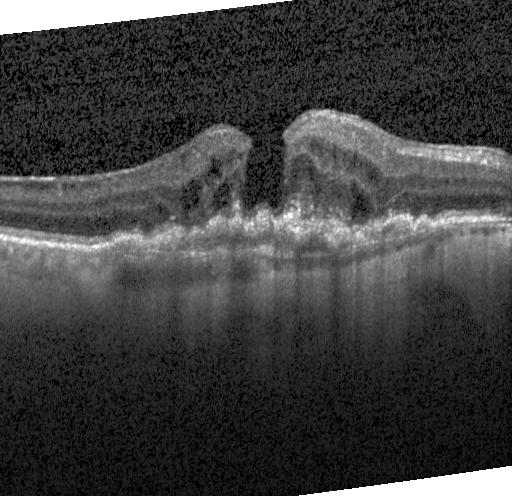

The scan shows a choroidal neovascular membrane.